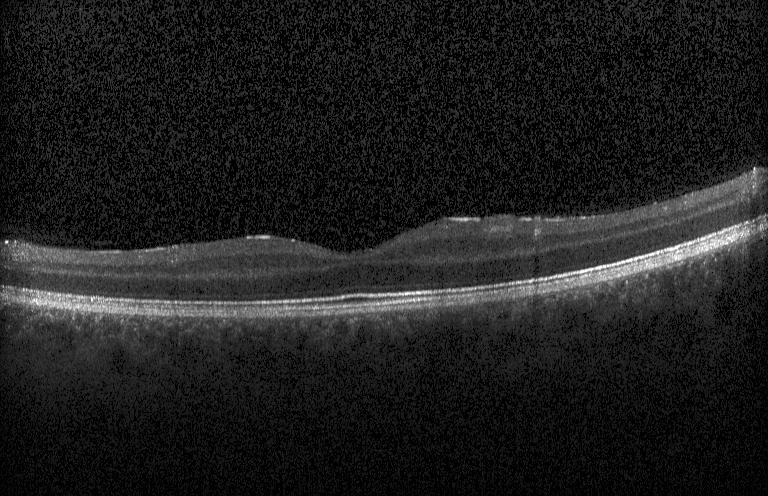 Optical coherence tomography B-scan; Heidelberg Spectralis OCT system — Dx: no choroidal neovascularization, no diabetic macular edema, and no drusen.